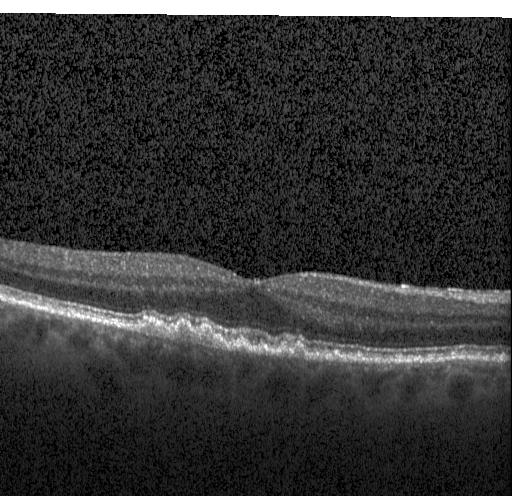

OCT B-scan. Diagnosis: multiple drusen.